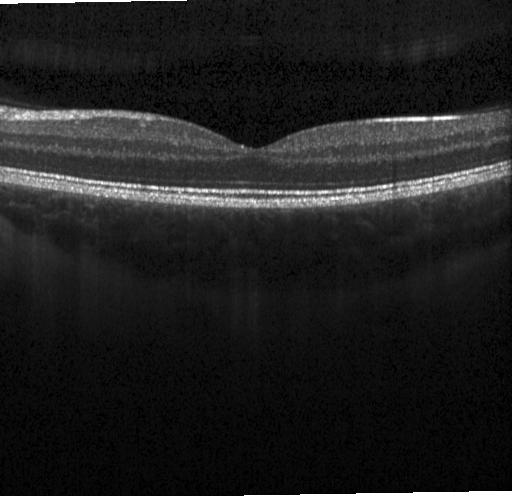

Optical coherence tomography scan, spectral-domain OCT, acquired on a Heidelberg Spectralis, through the macula.
Dx: no CNV, no DME, and no drusen.